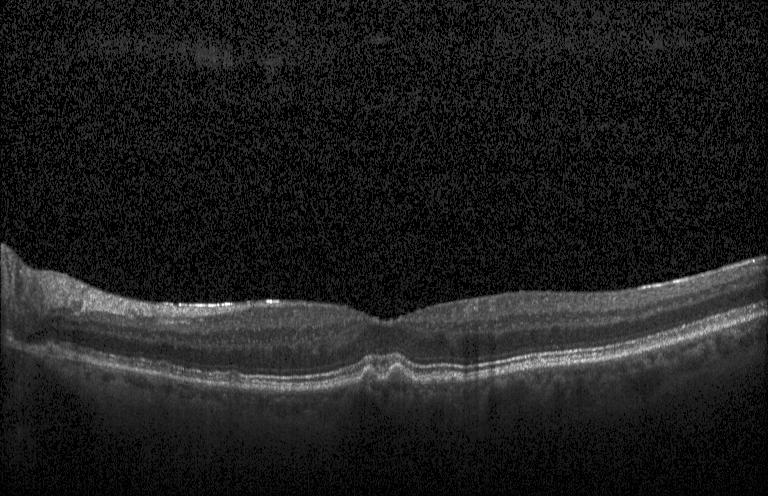 Spectral-domain OCT. OCT B-scan. Acquired on a Heidelberg Spectralis. Diagnosis: multiple drusen.